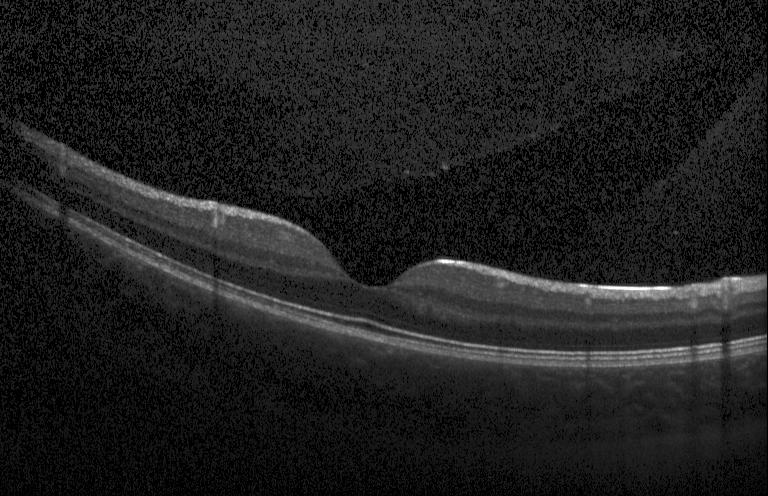 OCT line scan. Finding: neither CNV, DME, nor drusen.